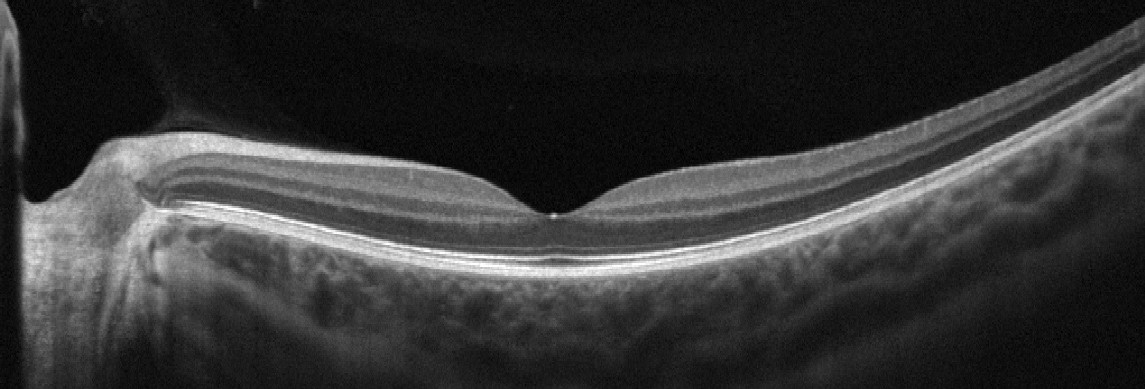
The scan shows no evidence of AMD, DME, ERM, RAO, RVO, or VID.